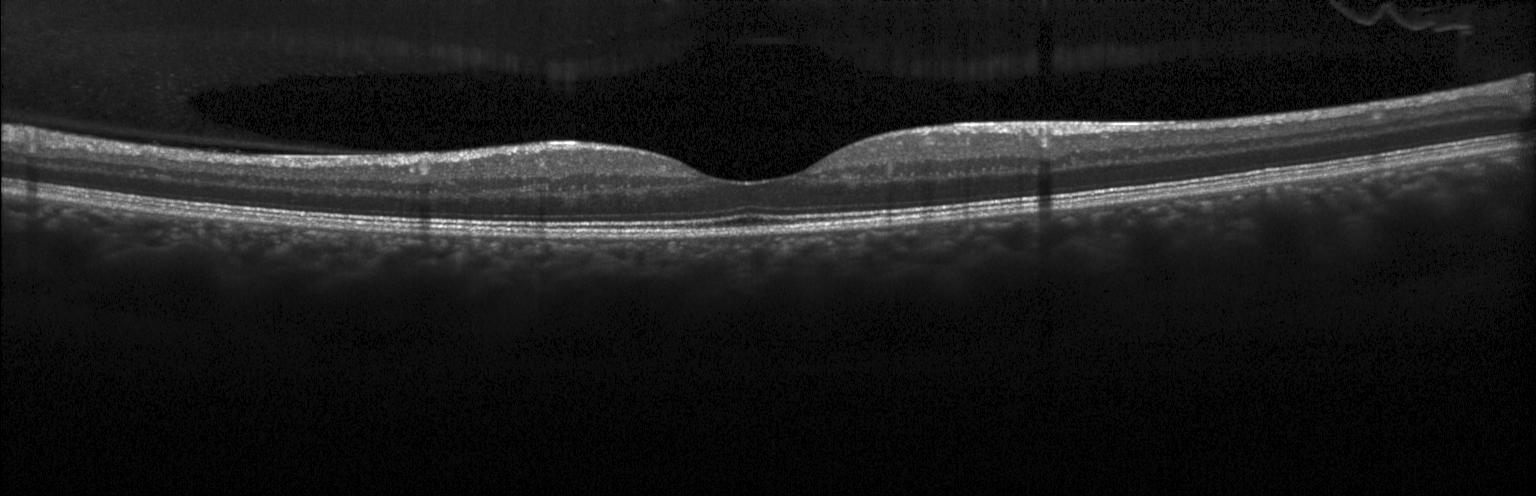

Assessment: no evidence of CNV, DME, or drusen.